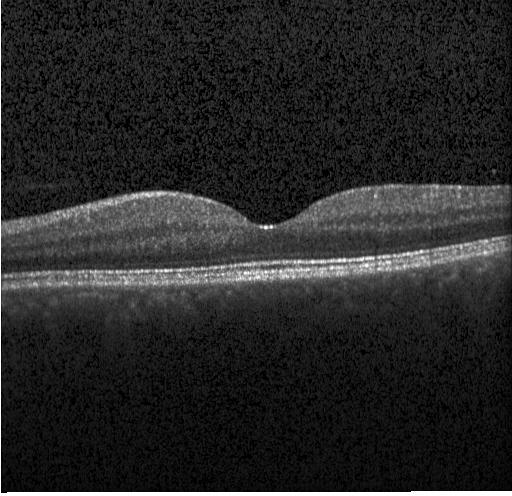
This B-scan demonstrates no evidence of CNV, DME, or drusen.